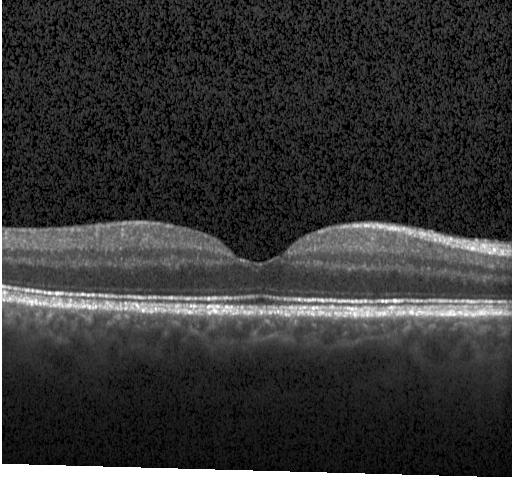

Macular OCT demonstrating no evidence of choroidal neovascularization, diabetic macular edema, or drusen.